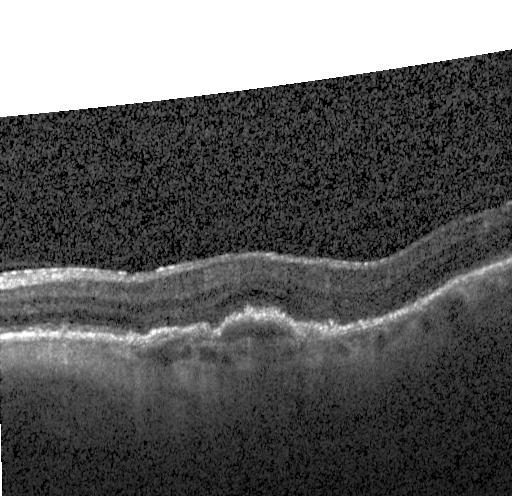 This B-scan demonstrates CNV.